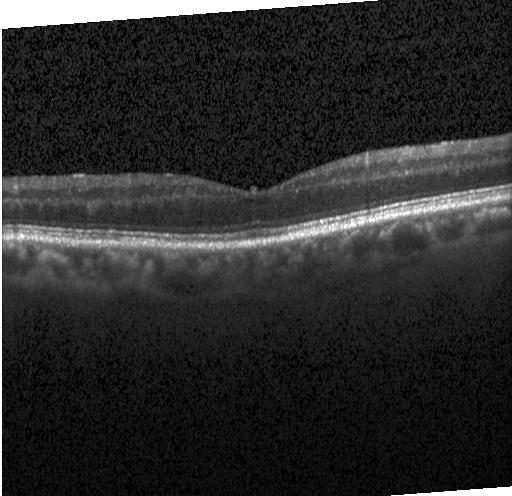

Macular OCT: no evidence of CNV, DME, or drusen.